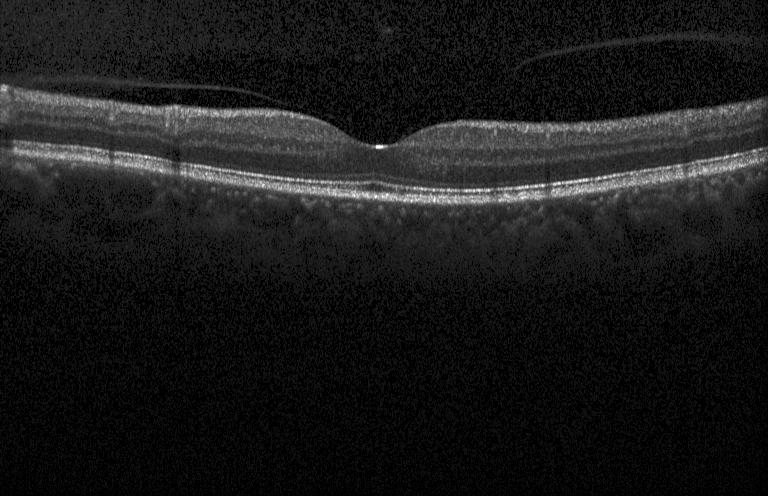

Dx: no choroidal neovascularization, no diabetic macular edema, and no drusen.